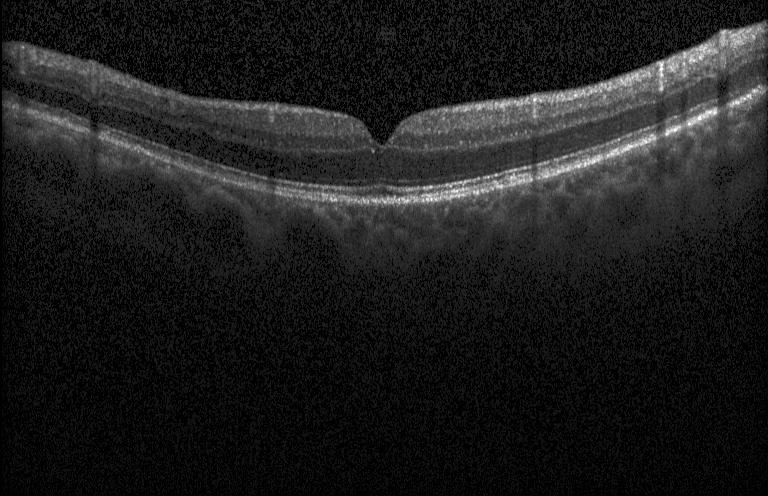
Diagnosis: no evidence of choroidal neovascularization, diabetic macular edema, or drusen.